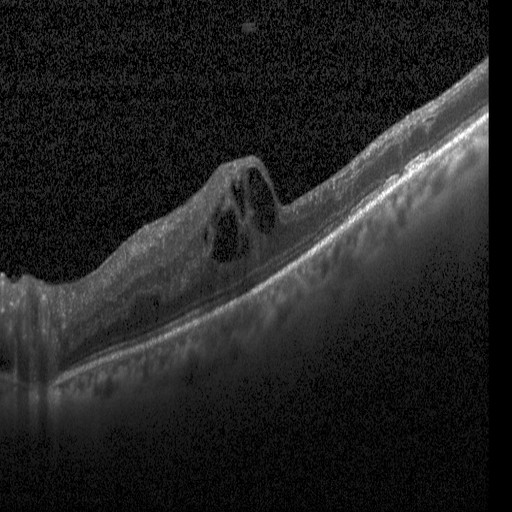
OCT line scan — Finding: DME.